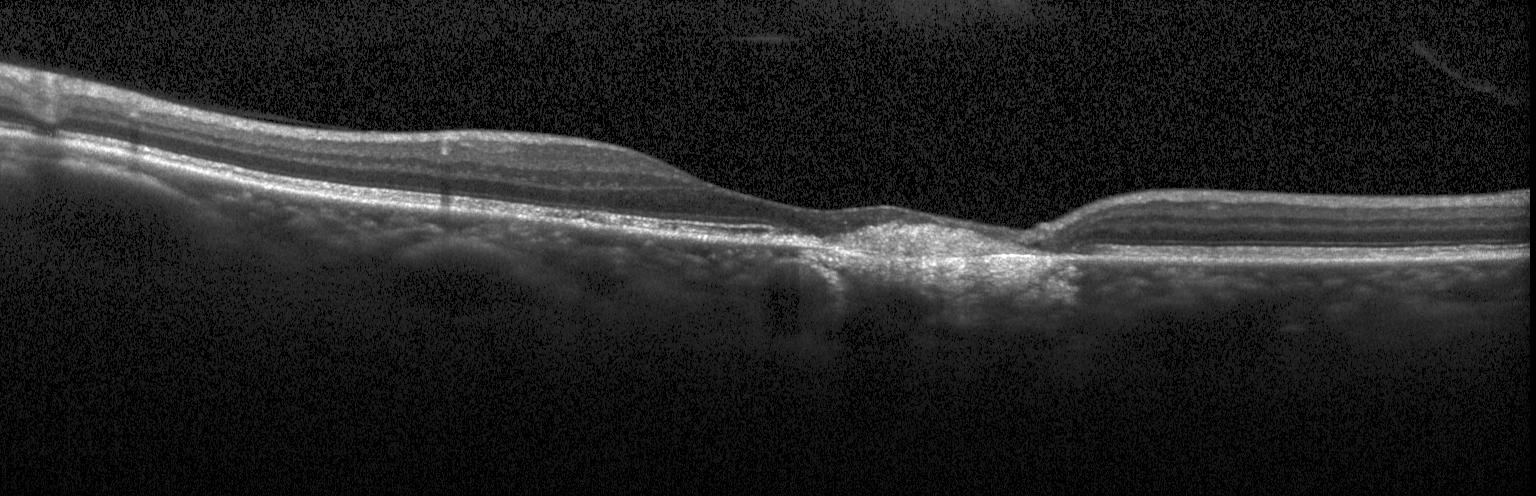

Spectral-domain OCT B-scan: a choroidal neovascular membrane.